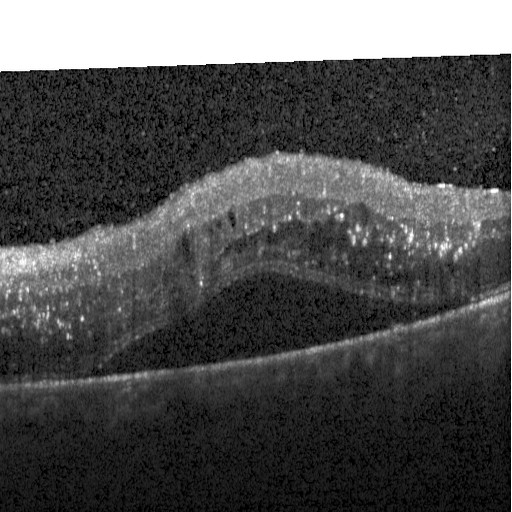

Retinal OCT cross-section, spectral-domain OCT, instrument: Heidelberg Spectralis, horizontal scan through the fovea
Macular OCT: DME.